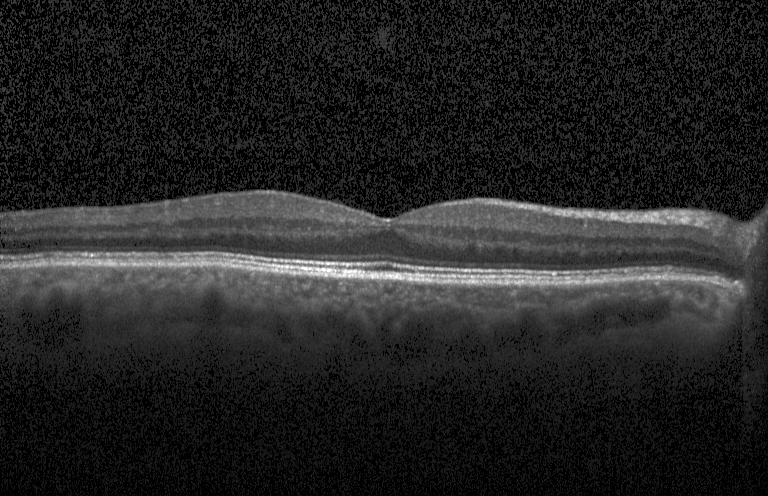 Finding: no choroidal neovascularization, no diabetic macular edema, and no drusen.